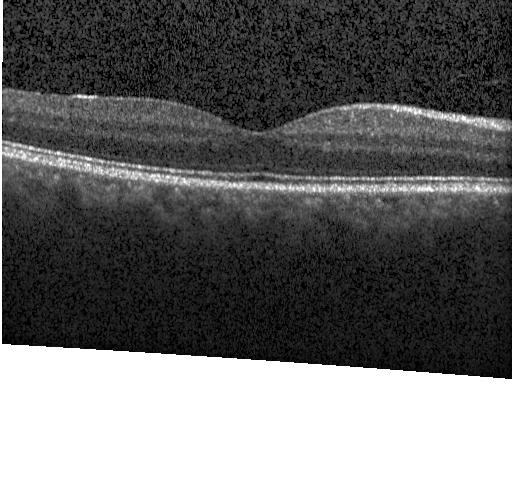
Instrument: Heidelberg Spectralis, centered on the fovea, optical coherence tomography B-scan.
Diagnosis: neither choroidal neovascularization, diabetic macular edema, nor drusen.